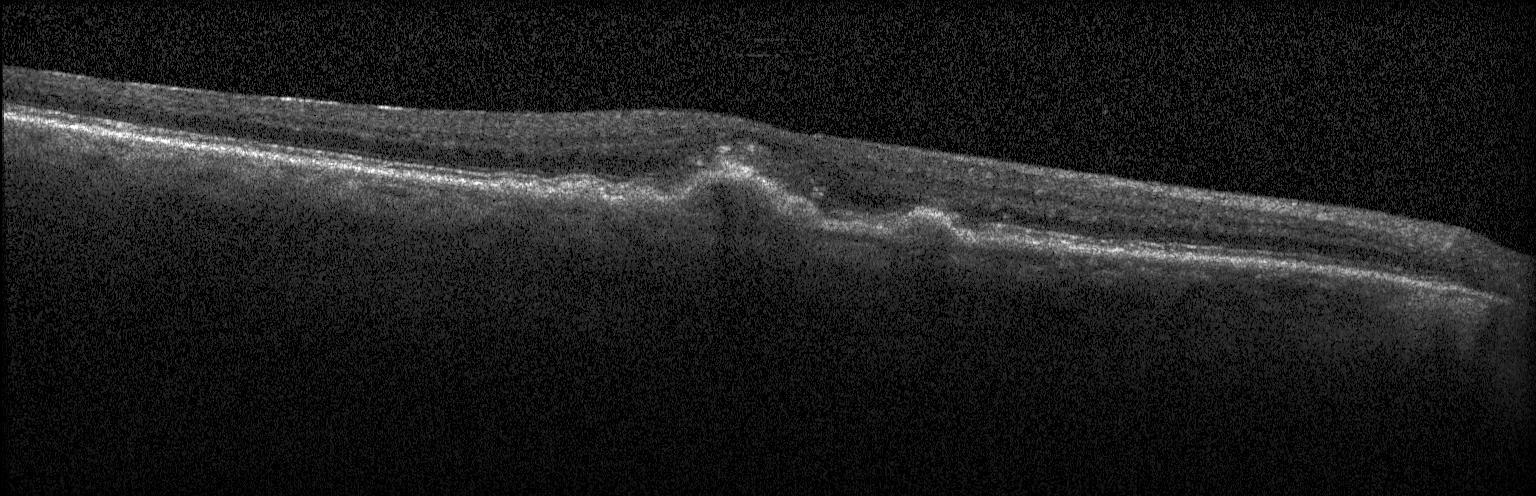

Optical coherence tomography scan
OCT finding: choroidal neovascularization (CNV).